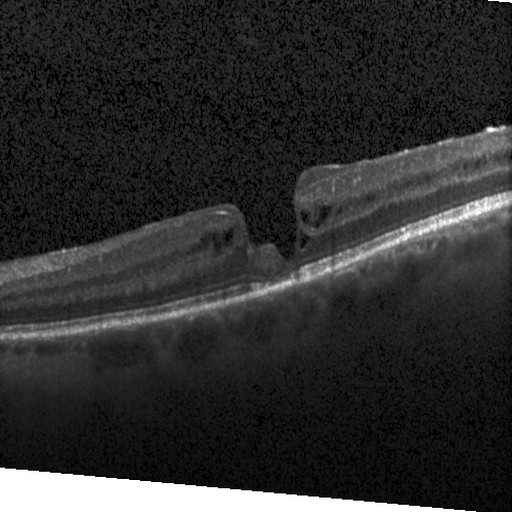 Finding: DME.